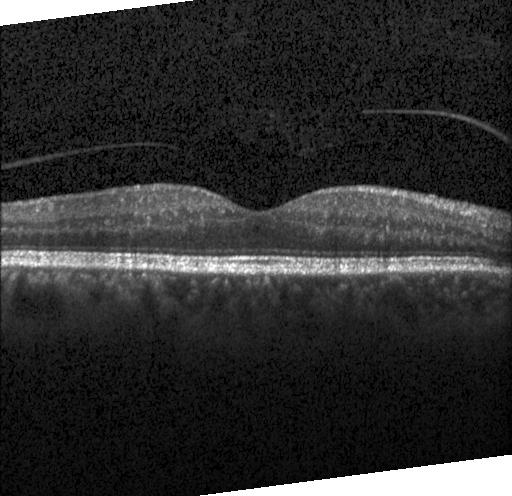 This B-scan demonstrates neither CNV, DME, nor drusen.